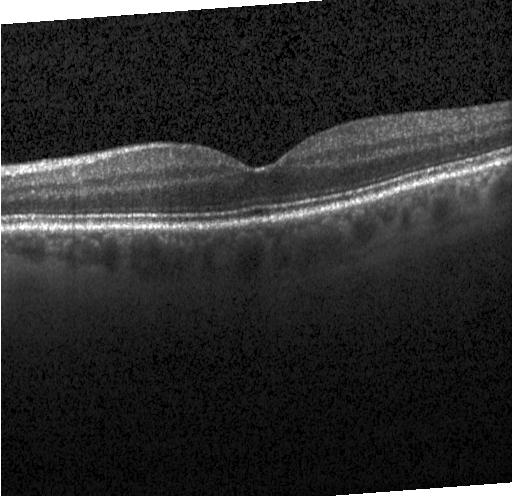
No choroidal neovascularization, no diabetic macular edema, and no drusen.